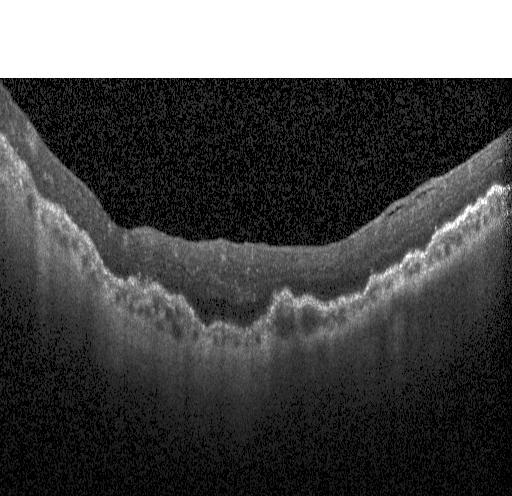

Assessment: a choroidal neovascular membrane.